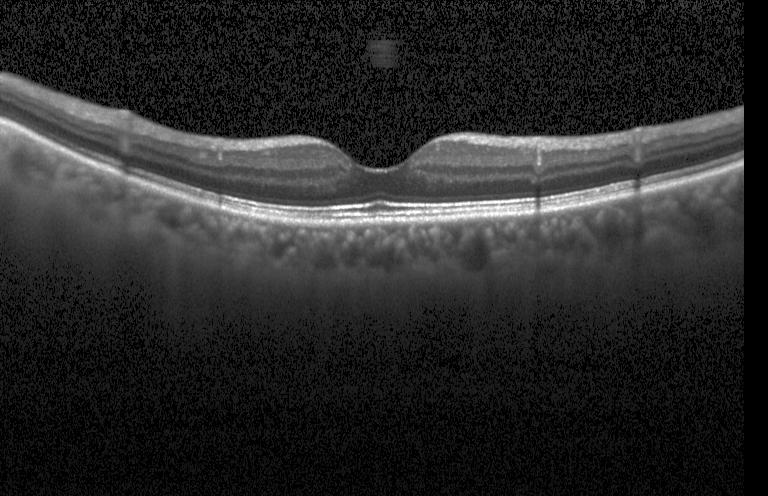 Heidelberg Spectralis; optical coherence tomography scan; spectral-domain OCT; fovea-centered
Assessment: no evidence of choroidal neovascularization, diabetic macular edema, or drusen.